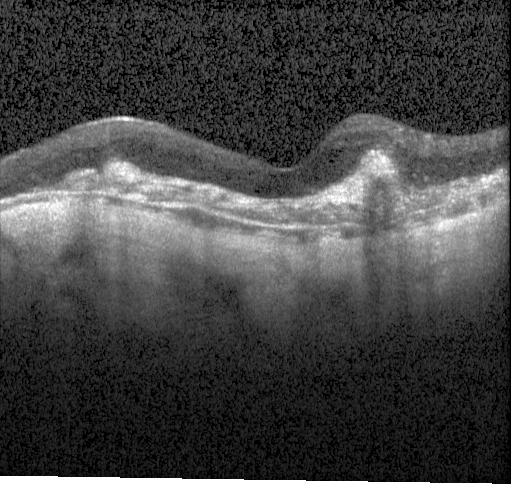

Spectral-domain optical coherence tomography. Acquired on a Heidelberg Spectralis. OCT line scan
The scan shows choroidal neovascularization.